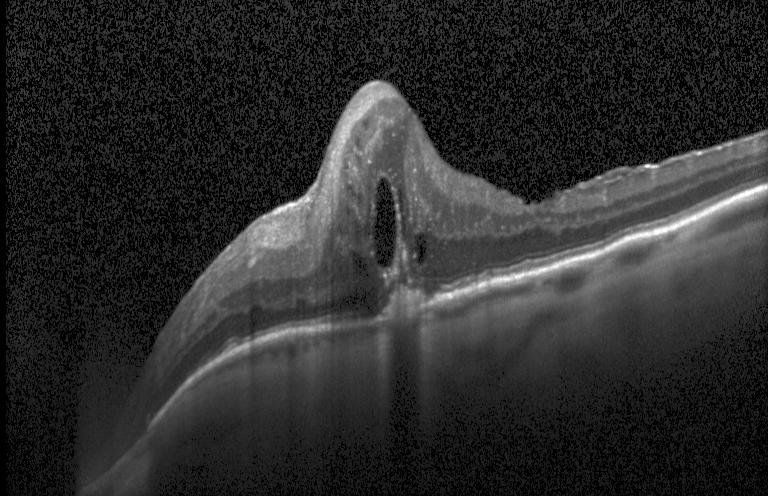 Macular OCT: choroidal neovascularization (CNV).